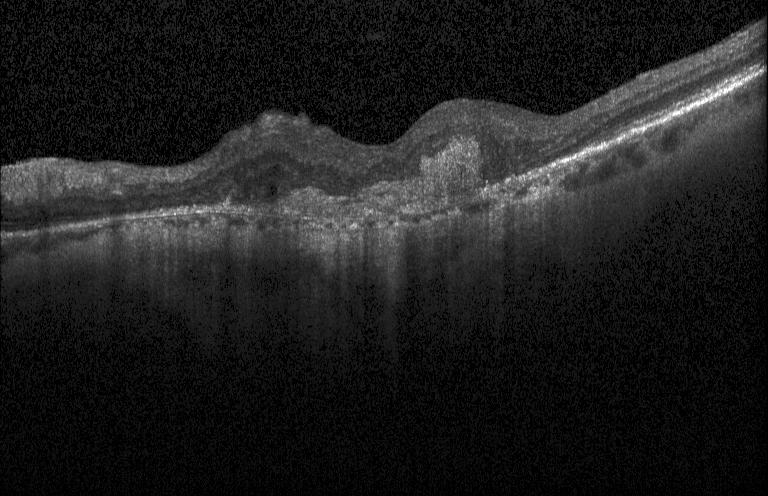 Finding: choroidal neovascularization.